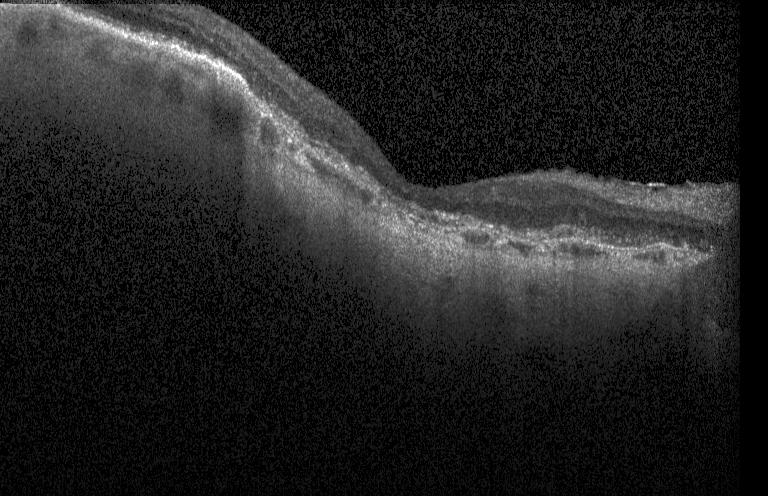

The scan shows a choroidal neovascular membrane.